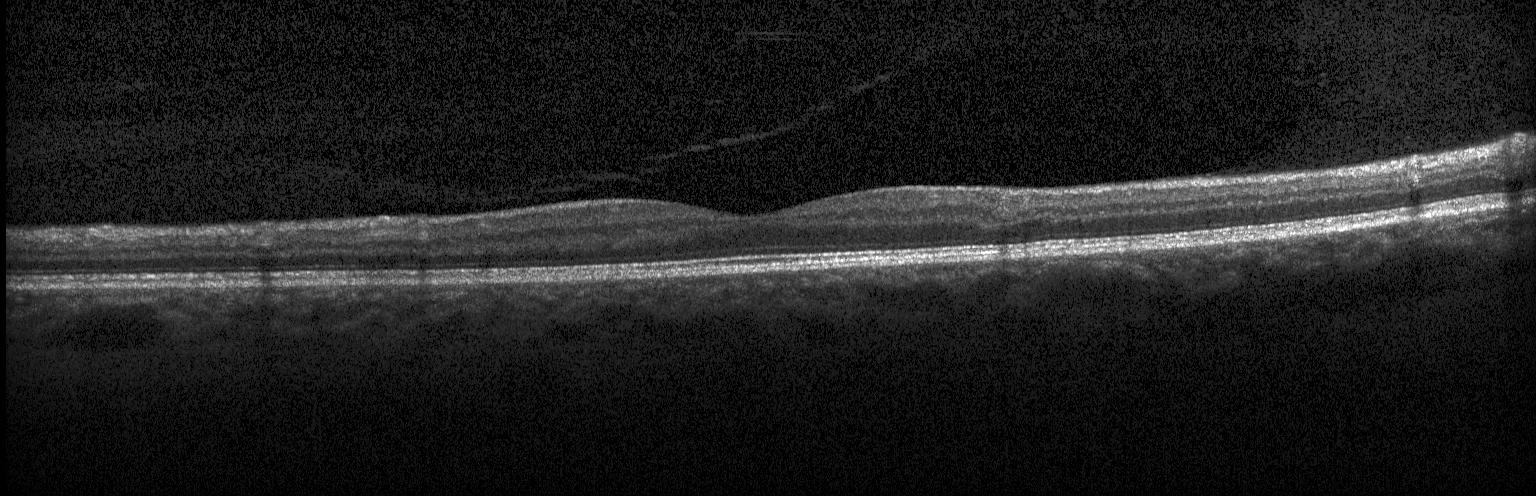 This B-scan demonstrates no choroidal neovascularization, no diabetic macular edema, and no drusen.